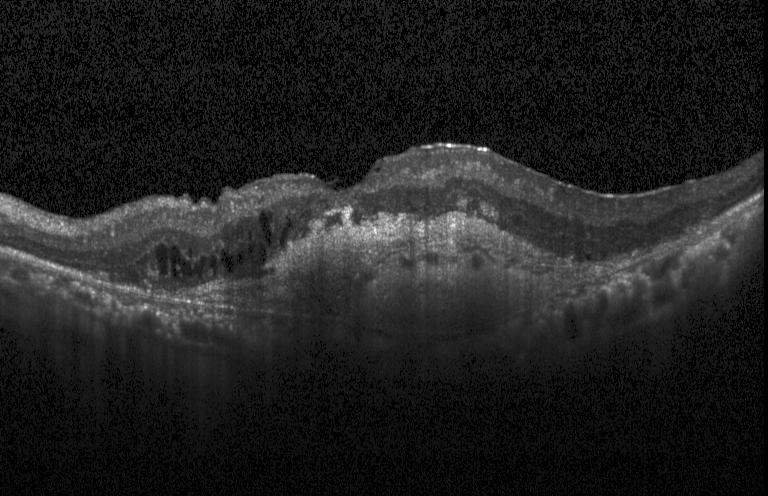
Dx: choroidal neovascularization (CNV).